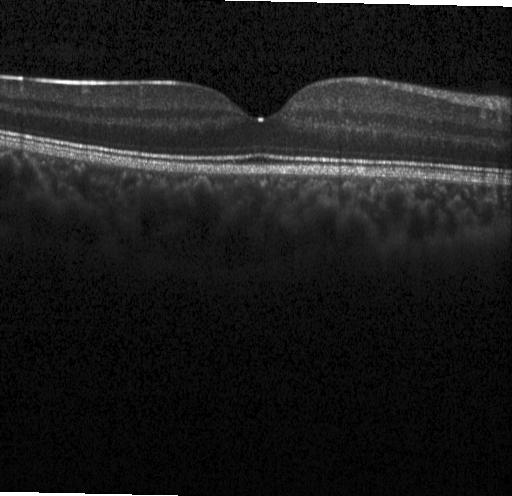
No choroidal neovascularization, diabetic macular edema, or drusen.